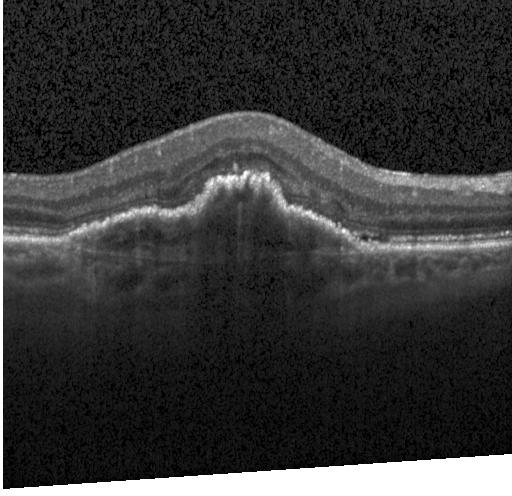
Macular scan; retinal OCT cross-section; acquired on a Heidelberg Spectralis; spectral-domain OCT.
Finding: choroidal neovascularization.